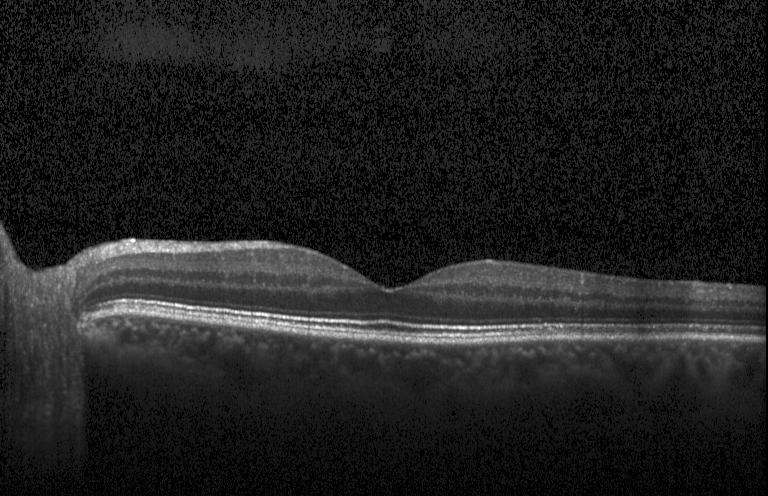 Fovea-centered · OCT B-scan — Impression: neither choroidal neovascularization, diabetic macular edema, nor drusen.